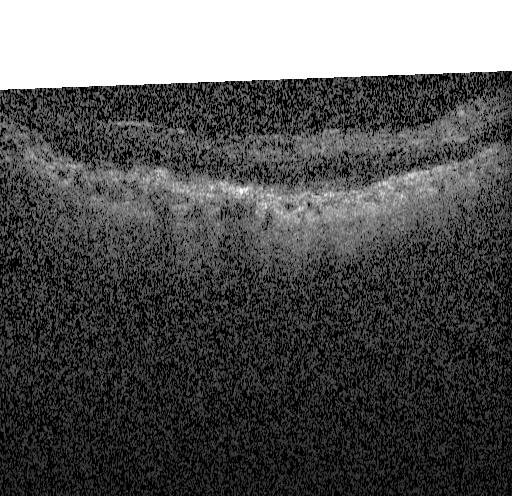 The scan shows CNV.